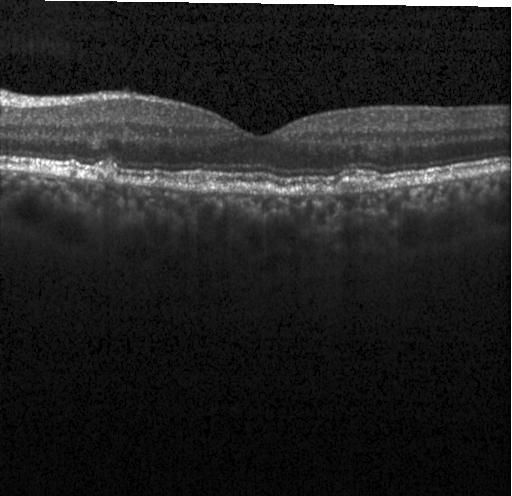
Diagnosis: multiple drusen.